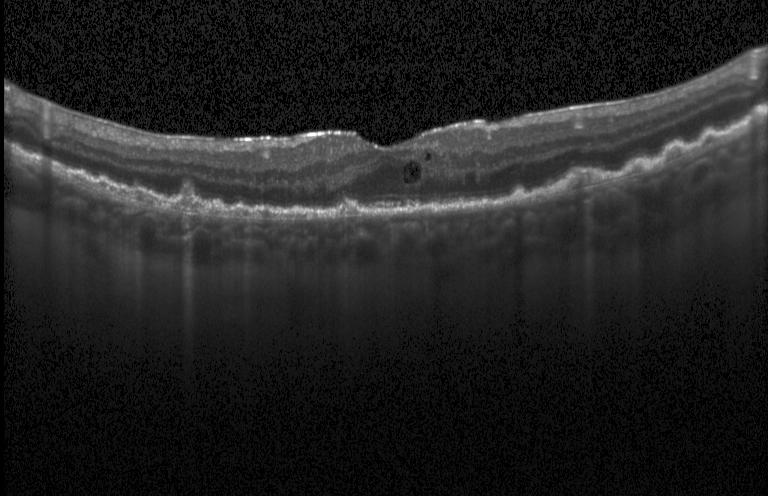

Heidelberg Spectralis; OCT B-scan; spectral-domain optical coherence tomography. Diagnosis: a choroidal neovascular membrane.